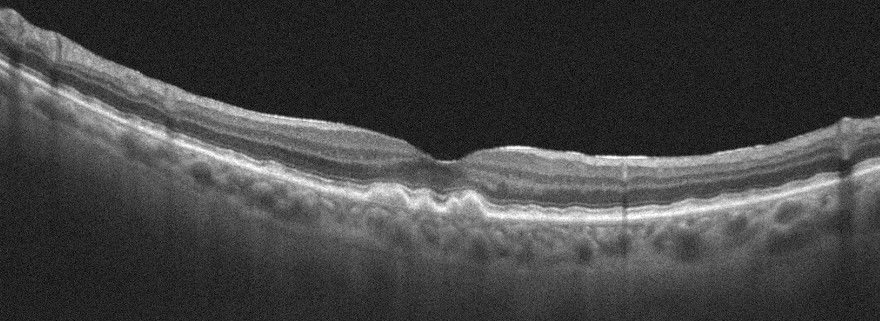
Optical coherence tomography B-scan. Finding: age-related macular degeneration (AMD).